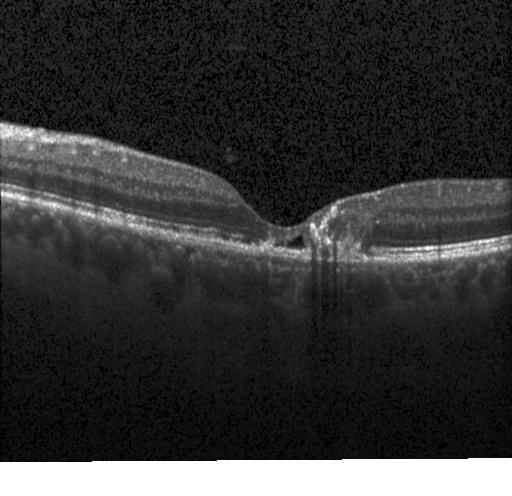
Macular OCT: a choroidal neovascular membrane.